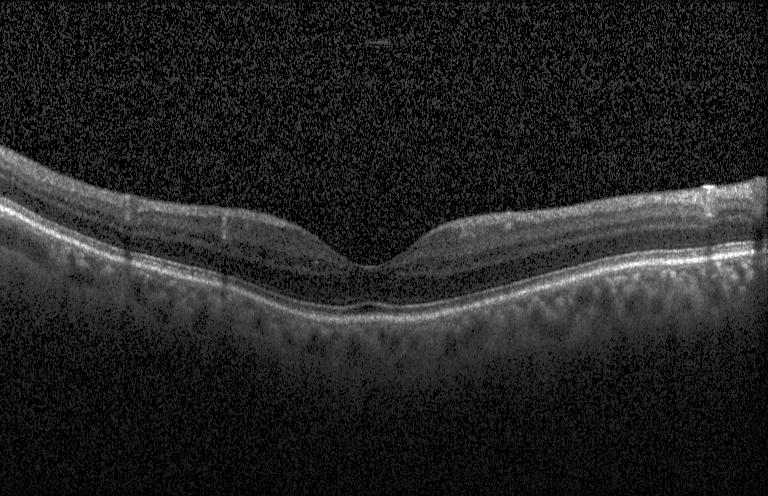 Macular OCT: no choroidal neovascularization, no diabetic macular edema, and no drusen.